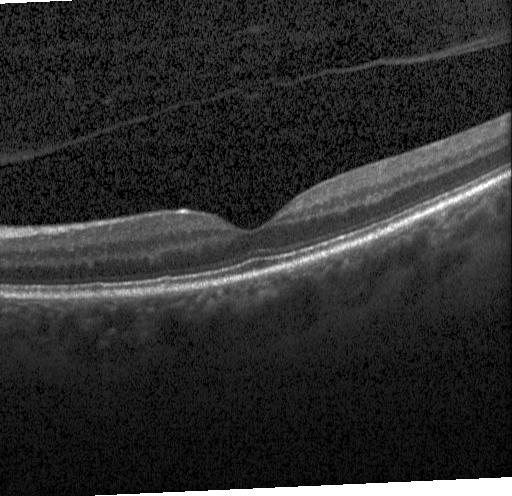
Optical coherence tomography B-scan · acquired on a Heidelberg Spectralis
Assessment: neither choroidal neovascularization, diabetic macular edema, nor drusen.